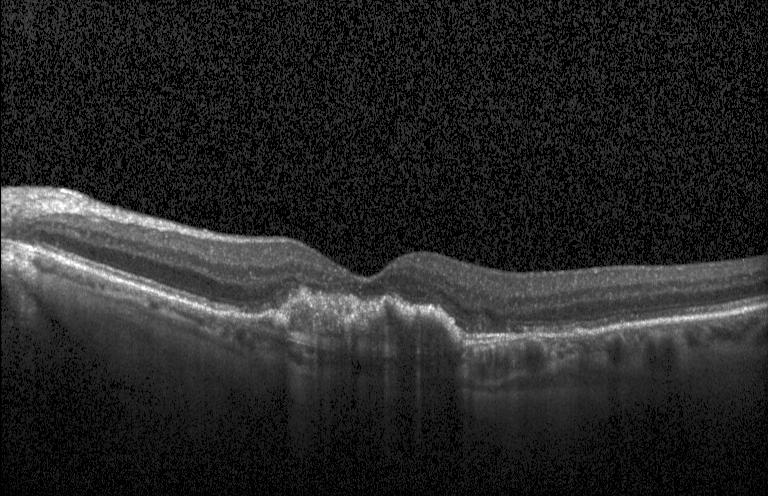
This B-scan demonstrates a choroidal neovascular membrane.